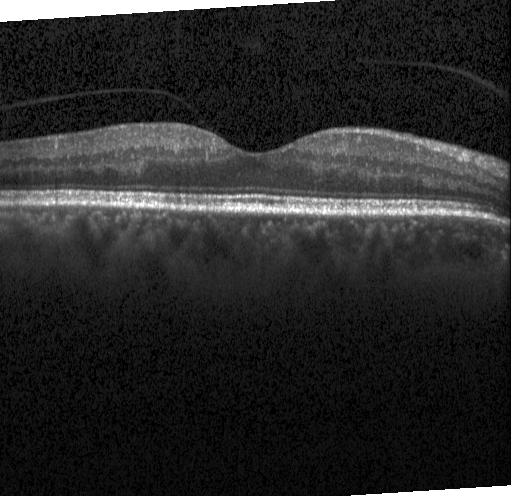
Diagnosis: no CNV, no DME, and no drusen.